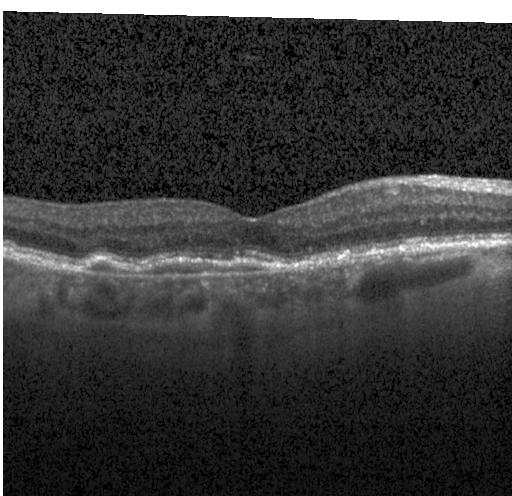

A choroidal neovascular membrane.